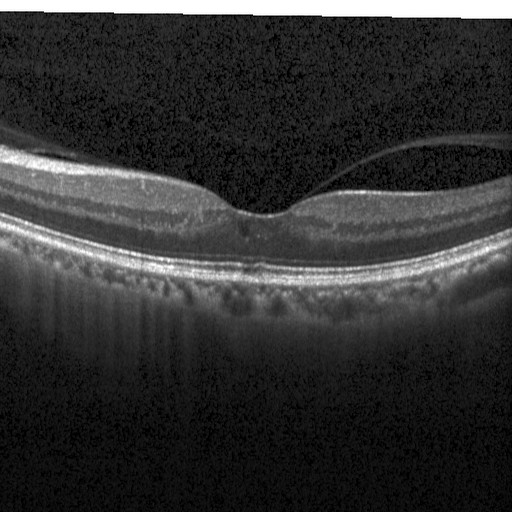
Dx: DME.